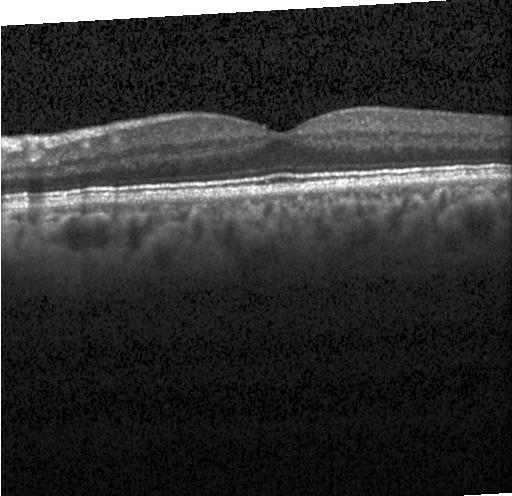 Fovea-centered · Heidelberg Spectralis · SD-OCT · OCT line scan
OCT finding: no choroidal neovascularization, diabetic macular edema, or drusen.